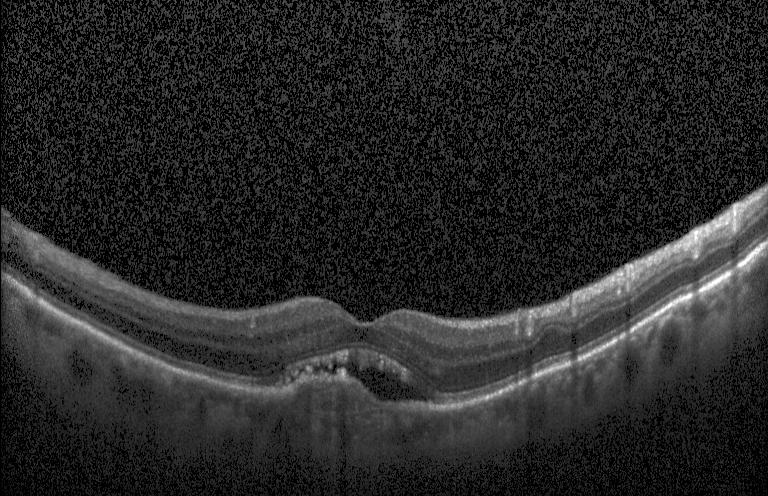 Heidelberg Spectralis OCT system; through the macula; spectral-domain OCT; retinal OCT cross-section — Impression: a choroidal neovascular membrane.